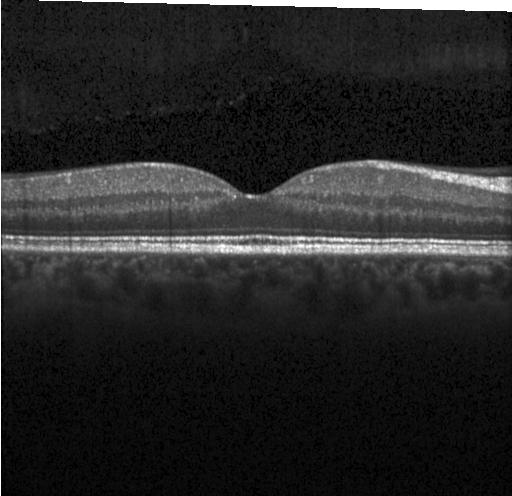 Horizontal scan through the fovea · optical coherence tomography B-scan.
This B-scan demonstrates no choroidal neovascularization, diabetic macular edema, or drusen.